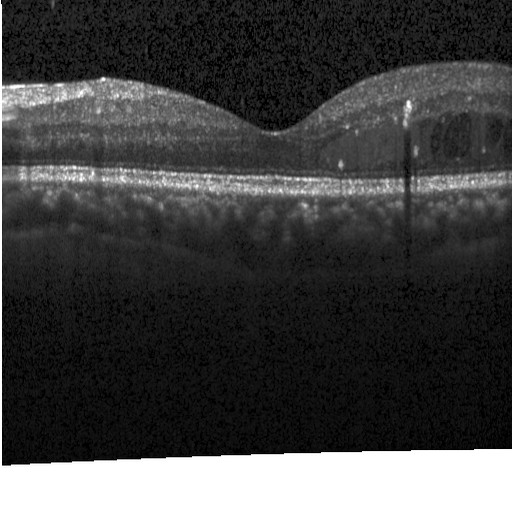 Optical coherence tomography scan. Centered on the fovea
DME.